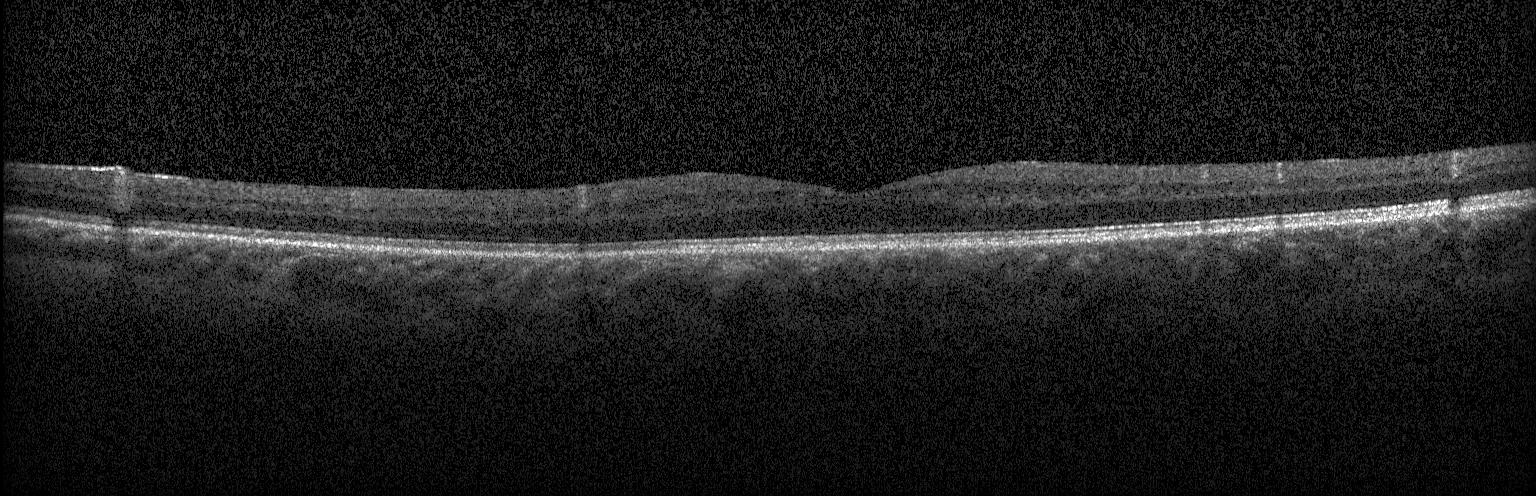 SD-OCT. Instrument: Heidelberg Spectralis. Centered on the fovea. Retinal OCT cross-section — Finding: neither choroidal neovascularization, diabetic macular edema, nor drusen.